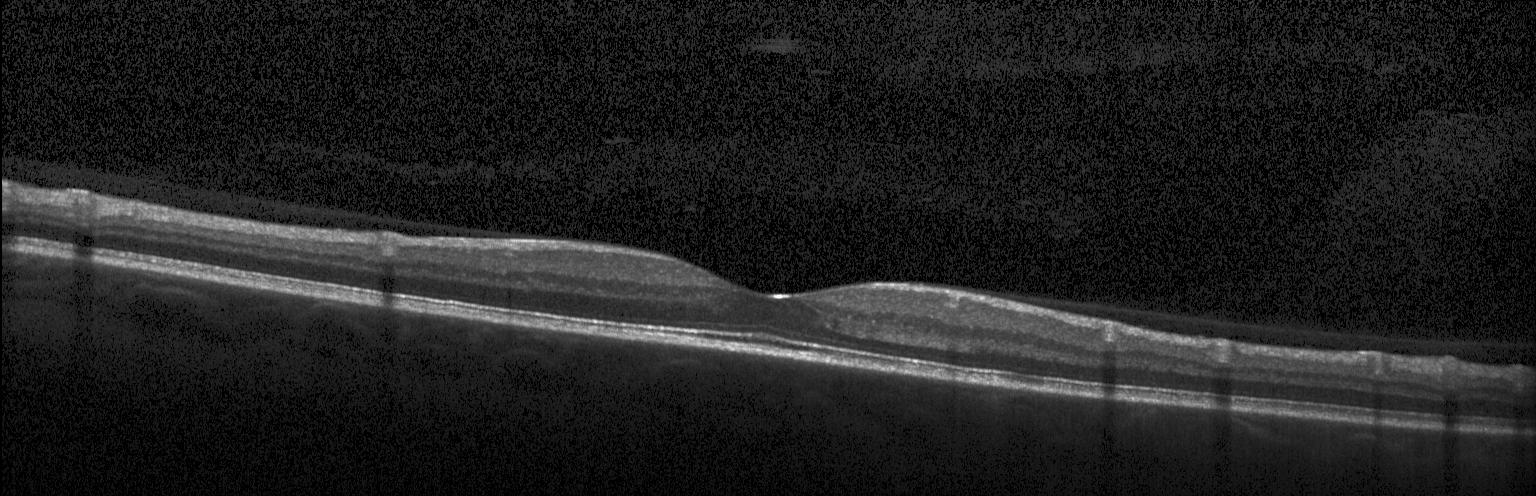 Retinal OCT B-scan · SD-OCT · instrument: Heidelberg Spectralis · centered on the fovea
Finding: no choroidal neovascularization, diabetic macular edema, or drusen.